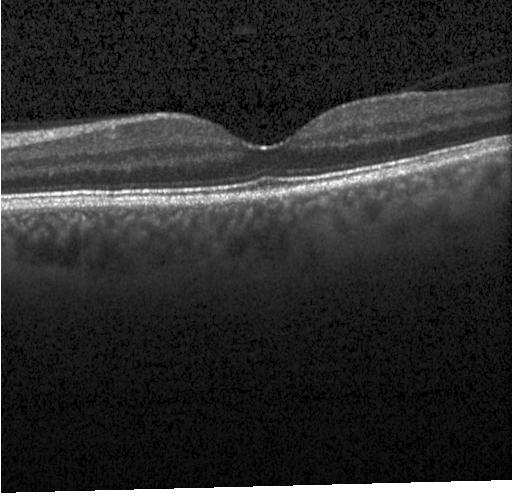
Optical coherence tomography scan. Macular scan. Acquired on a Heidelberg Spectralis. SD-OCT
No choroidal neovascularization, no diabetic macular edema, and no drusen.